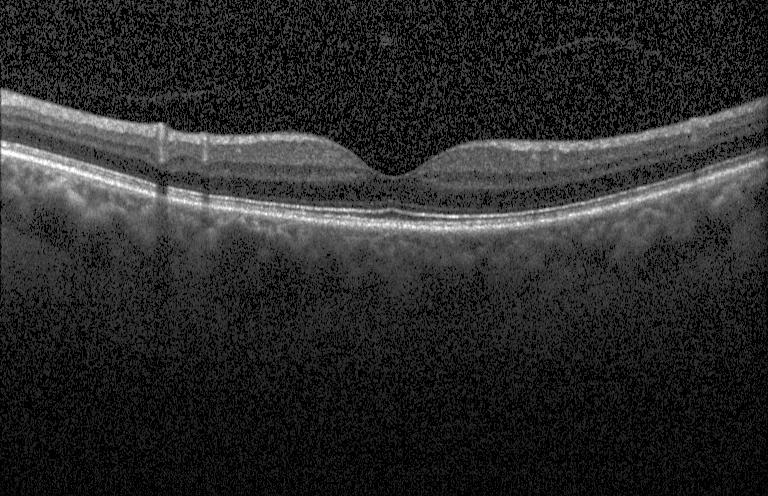 Optical coherence tomography scan; SD-OCT.
Finding: no evidence of choroidal neovascularization, diabetic macular edema, or drusen.